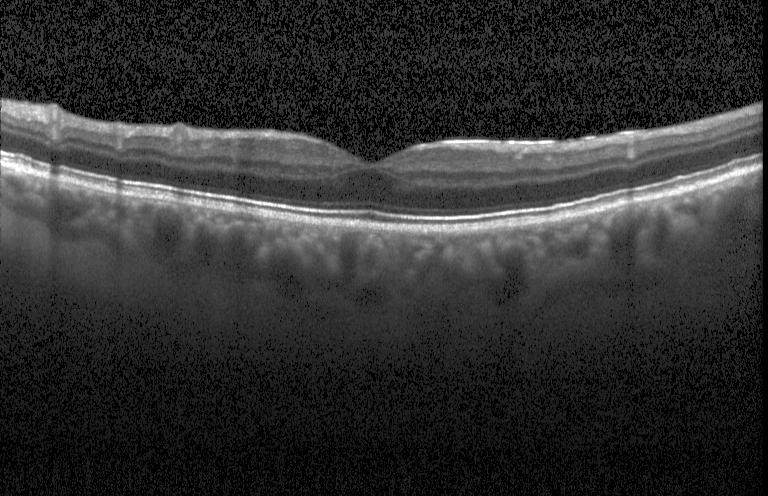
SD-OCT. Macular scan. Retinal OCT B-scan.
Diagnosis: no choroidal neovascularization, no diabetic macular edema, and no drusen.